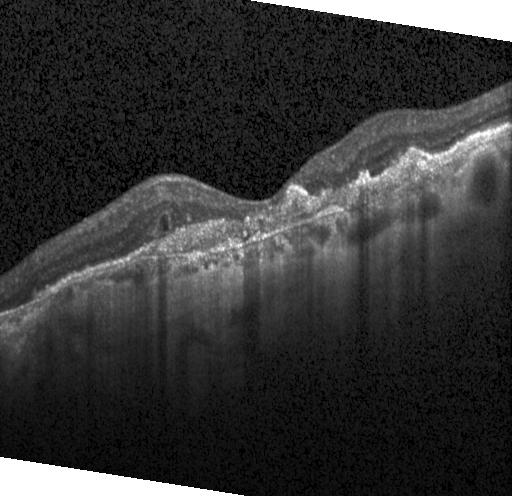

Fovea-centered; OCT B-scan; acquired on a Heidelberg Spectralis; spectral-domain OCT — Diagnosis: choroidal neovascularization.